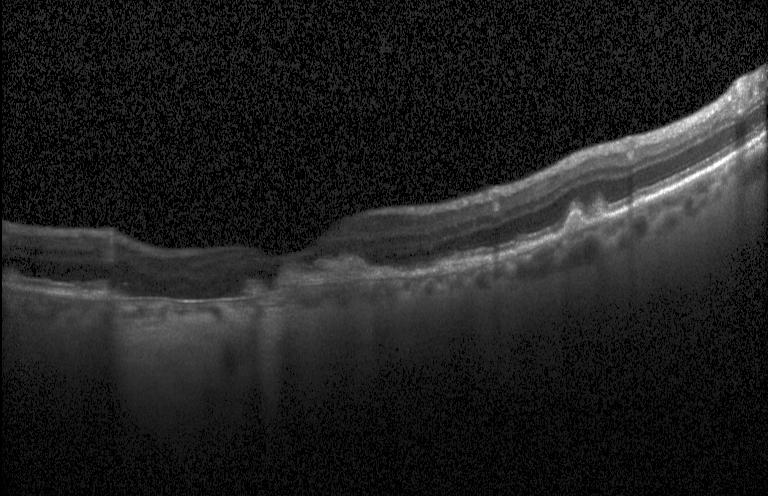 Retinal OCT B-scan.
Choroidal neovascularization (CNV).